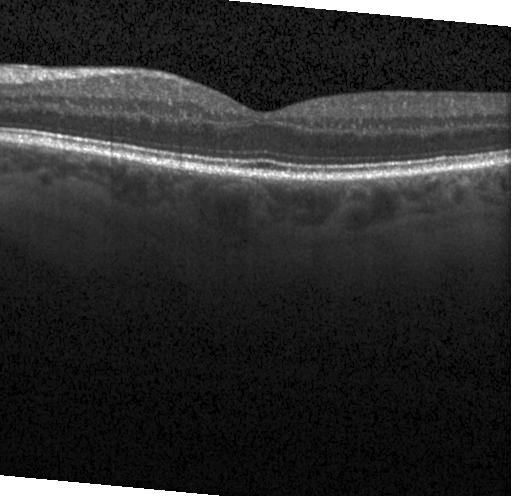

Finding: no choroidal neovascularization, diabetic macular edema, or drusen.